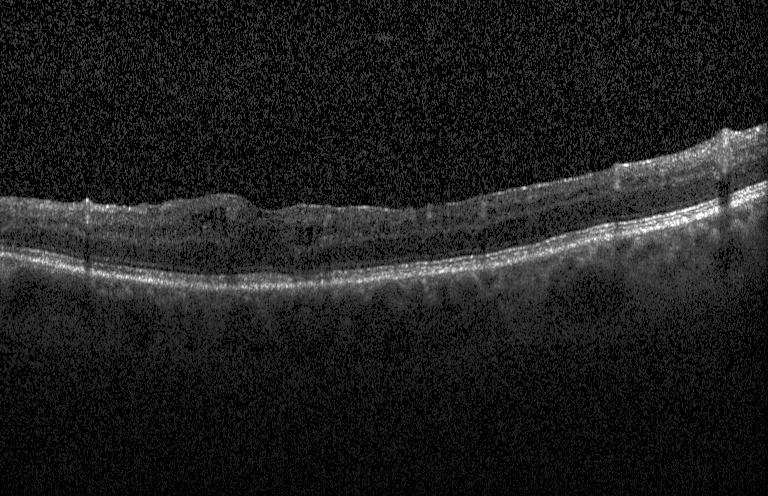
Fovea-centered; retinal OCT B-scan
Assessment: DME.